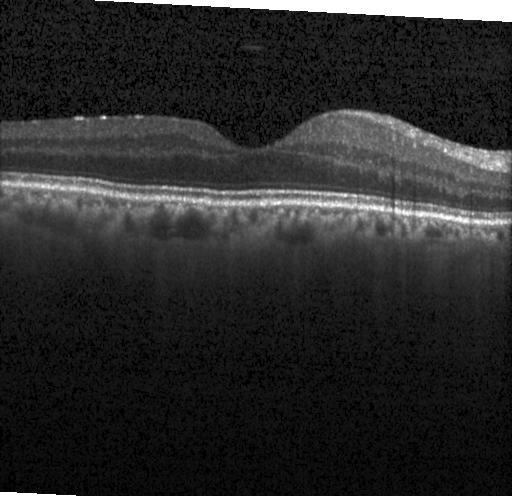 Retinal OCT cross-section, spectral-domain OCT.
Assessment: neither choroidal neovascularization, diabetic macular edema, nor drusen.